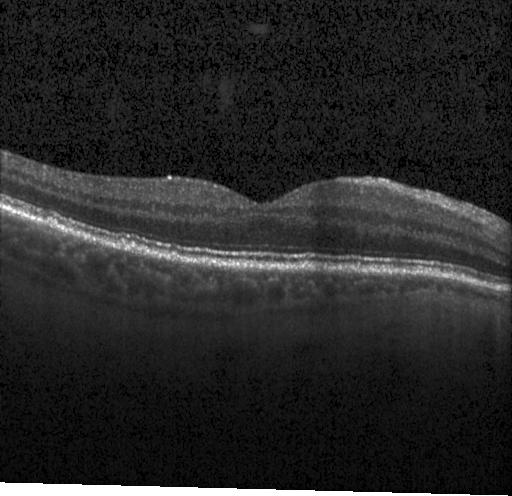
Fovea-centered; Heidelberg Spectralis; OCT B-scan; spectral-domain optical coherence tomography — Finding: multiple drusen.